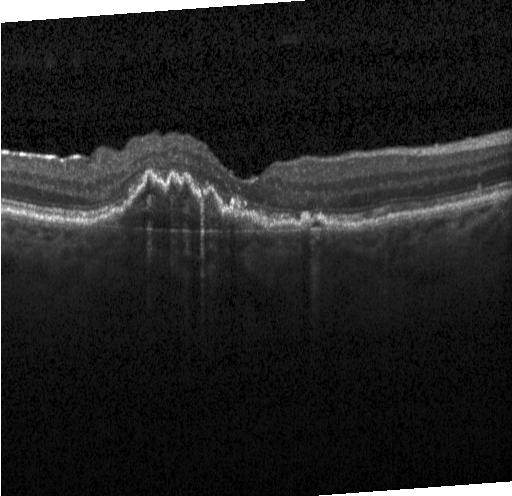
Instrument: Heidelberg Spectralis · retinal OCT B-scan · through the macula · SD-OCT. Impression: a choroidal neovascular membrane.